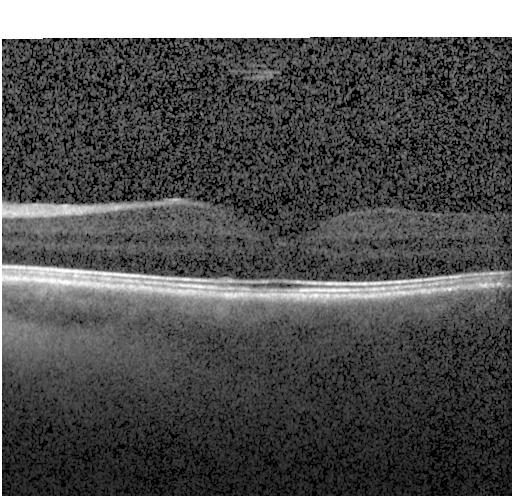 Heidelberg Spectralis OCT system, spectral-domain OCT, optical coherence tomography B-scan
Impression: no choroidal neovascularization, no diabetic macular edema, and no drusen.